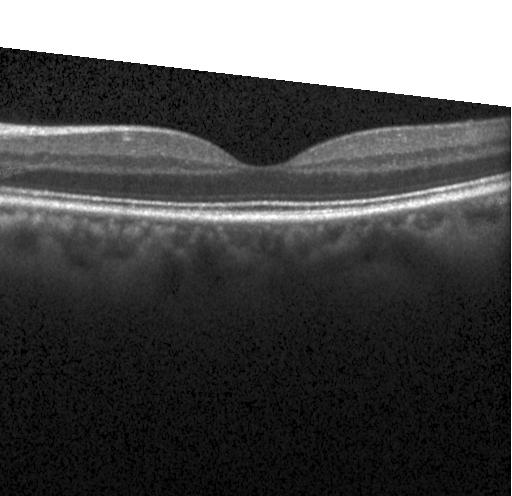

Optical coherence tomography B-scan.
Impression: neither choroidal neovascularization, diabetic macular edema, nor drusen.